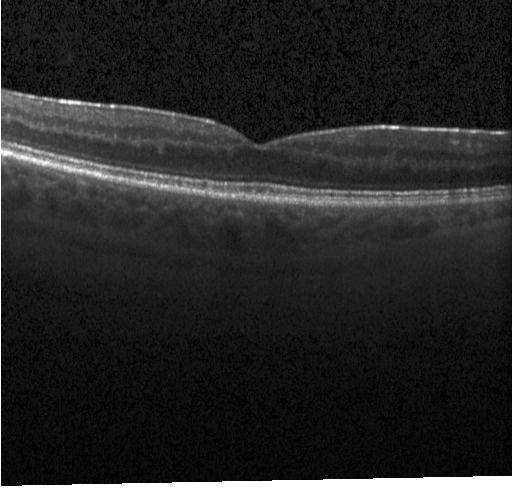
Optical coherence tomography scan.
Macular OCT: neither choroidal neovascularization, diabetic macular edema, nor drusen.